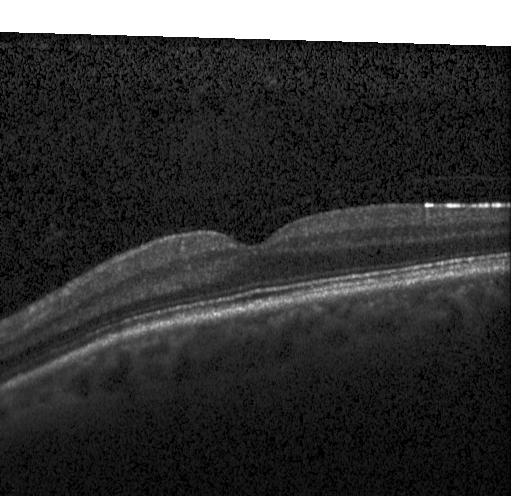

SD-OCT · acquired on a Heidelberg Spectralis · fovea-centered · optical coherence tomography B-scan.
This B-scan demonstrates neither choroidal neovascularization, diabetic macular edema, nor drusen.